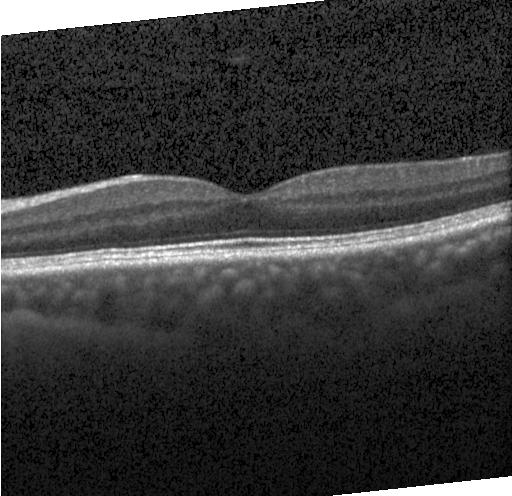

Optical coherence tomography scan, spectral-domain optical coherence tomography — Impression: no evidence of choroidal neovascularization, diabetic macular edema, or drusen.